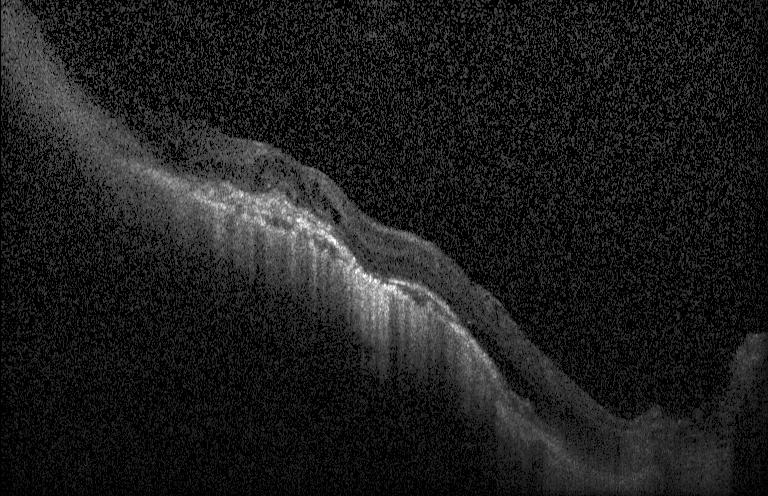

Impression: choroidal neovascularization.